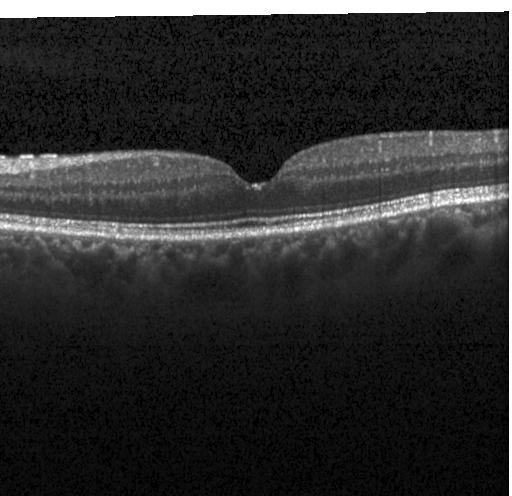

Diagnosis: no evidence of choroidal neovascularization, diabetic macular edema, or drusen.